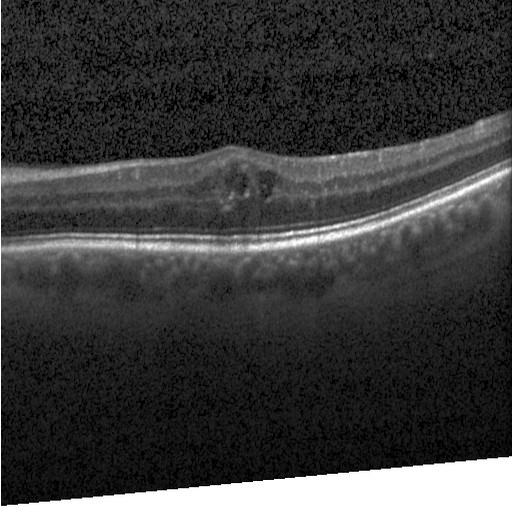
OCT line scan · instrument: Heidelberg Spectralis
Diagnosis: diabetic macular edema.